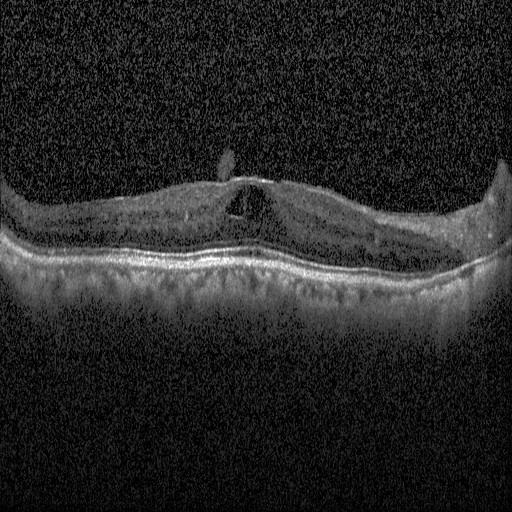 Optical coherence tomography B-scan; Heidelberg Spectralis OCT system; centered on the fovea; SD-OCT
Diabetic macular edema (DME).